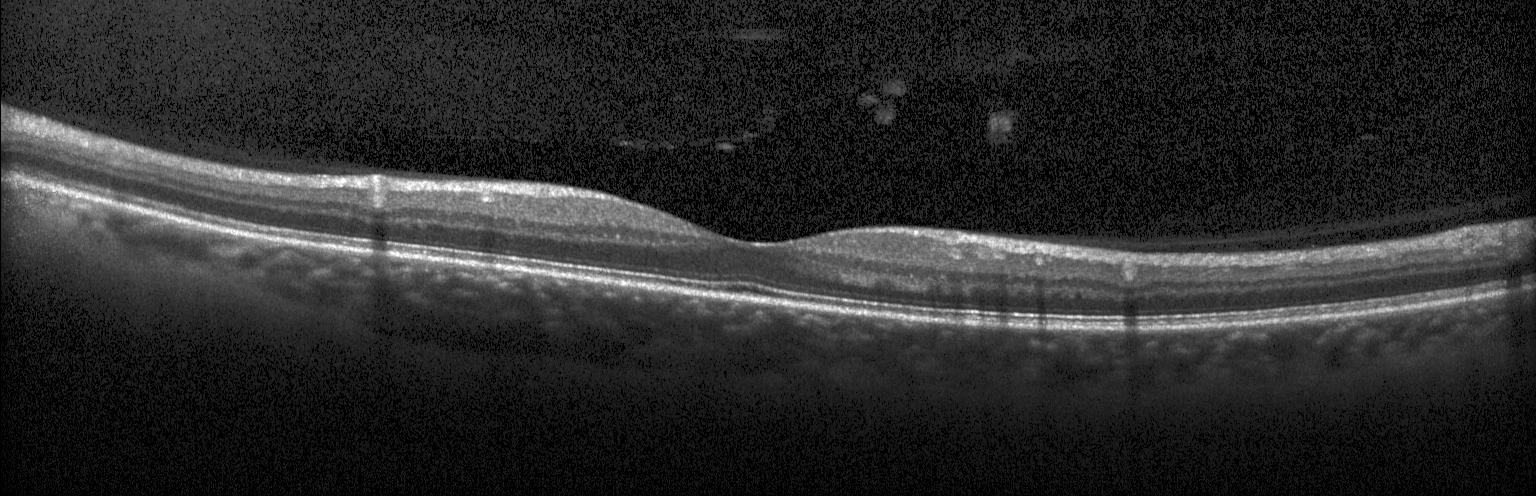
Acquired on a Heidelberg Spectralis, retinal OCT B-scan
Impression: no evidence of choroidal neovascularization, diabetic macular edema, or drusen.